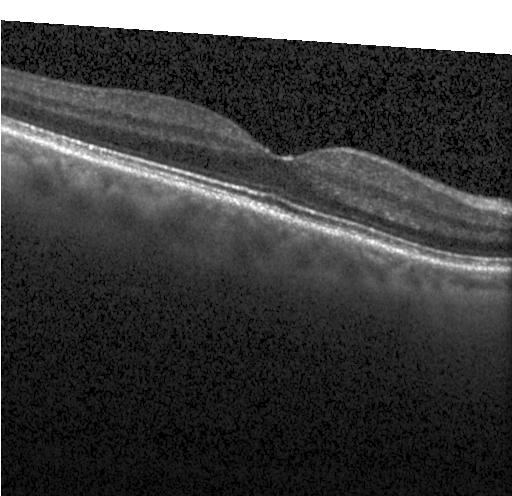
Macular scan; Heidelberg Spectralis OCT system; optical coherence tomography scan.
Finding: no evidence of choroidal neovascularization, diabetic macular edema, or drusen.